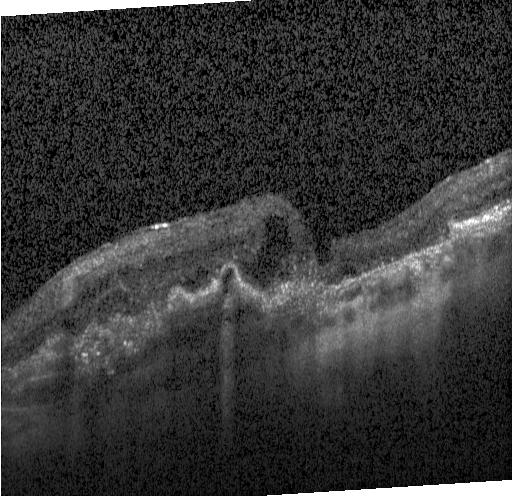

OCT scan showing a choroidal neovascular membrane.